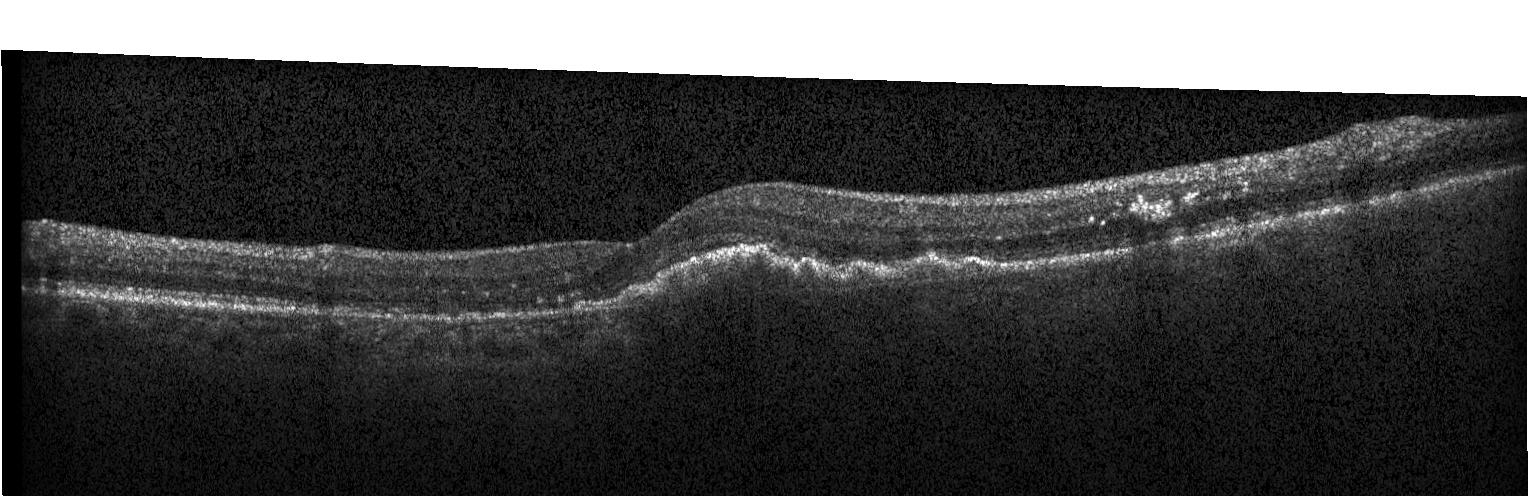 Optical coherence tomography B-scan · SD-OCT — OCT finding: CNV.